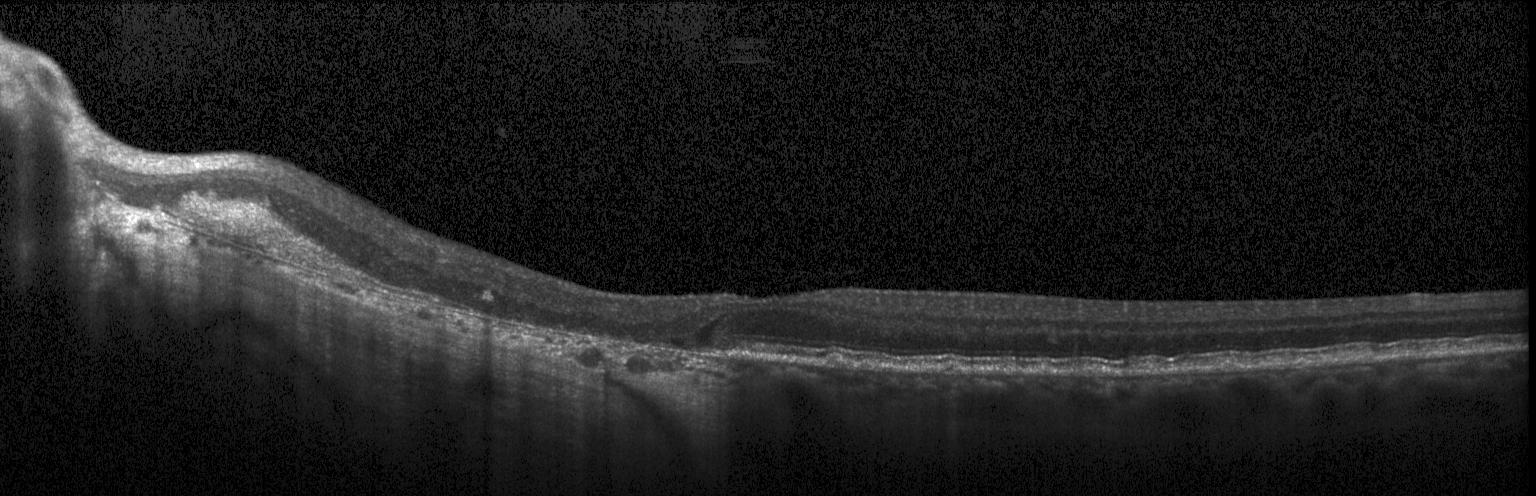

Spectral-domain OCT; optical coherence tomography scan
Assessment: CNV.